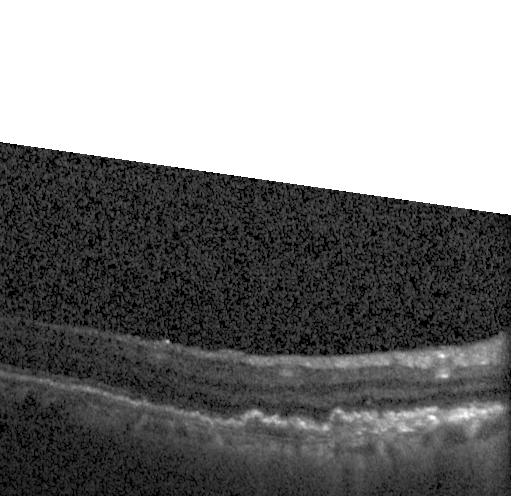 Impression: choroidal neovascularization.